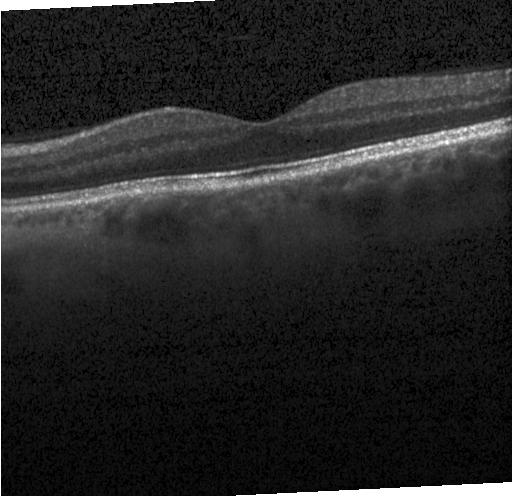
OCT line scan. Dx: no CNV, no DME, and no drusen.